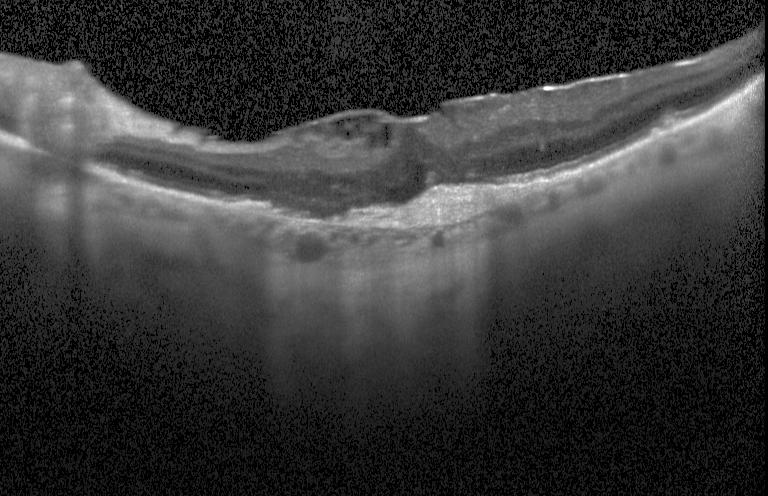 OCT B-scan showing a choroidal neovascular membrane.